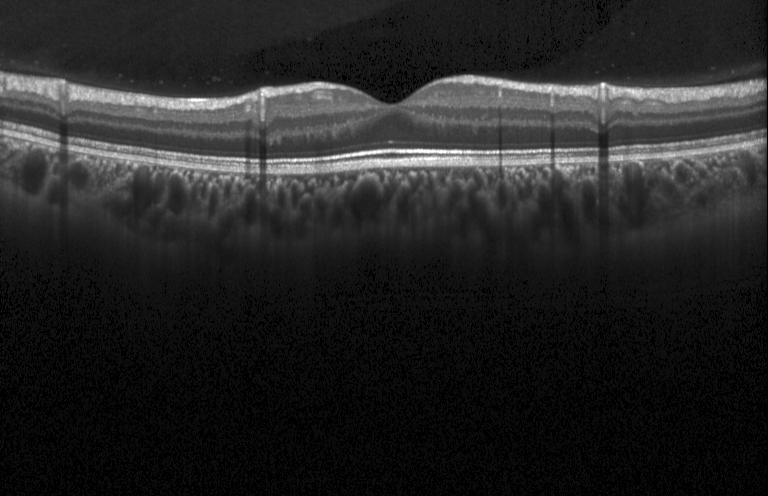

Finding: no choroidal neovascularization, diabetic macular edema, or drusen.